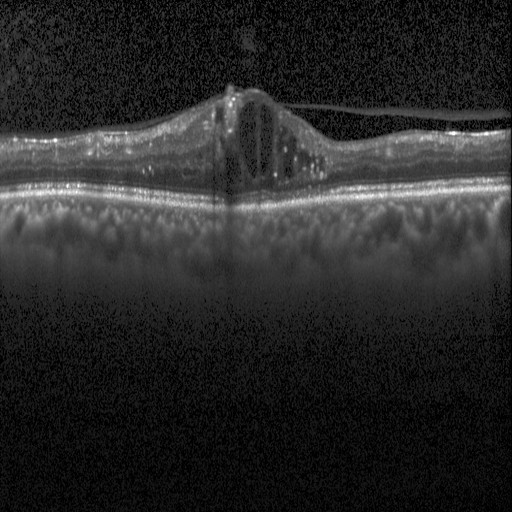 Impression: diabetic macular edema (DME).